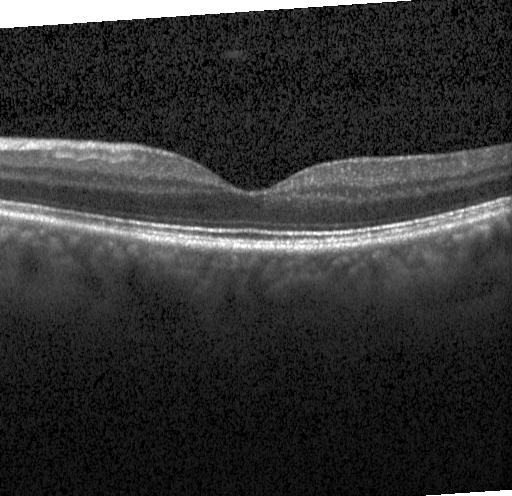 Heidelberg Spectralis OCT system. Optical coherence tomography B-scan
Macular OCT: no choroidal neovascularization, diabetic macular edema, or drusen.